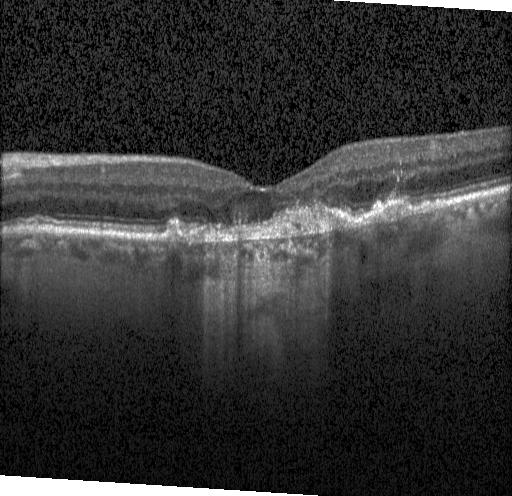

Heidelberg Spectralis; spectral-domain OCT; retinal OCT B-scan.
Finding: a choroidal neovascular membrane.